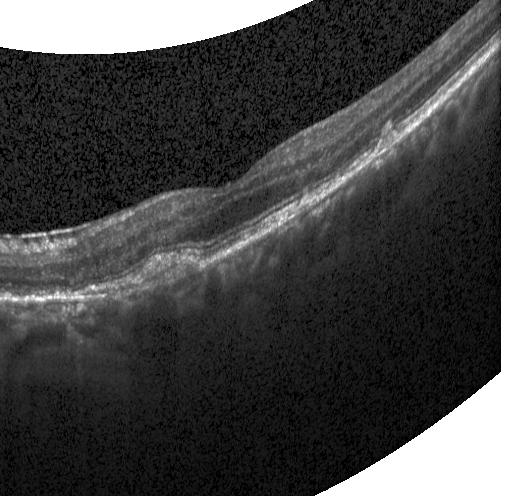

Centered on the fovea; spectral-domain OCT; acquired on a Heidelberg Spectralis; optical coherence tomography B-scan.
Diagnosis: choroidal neovascularization.